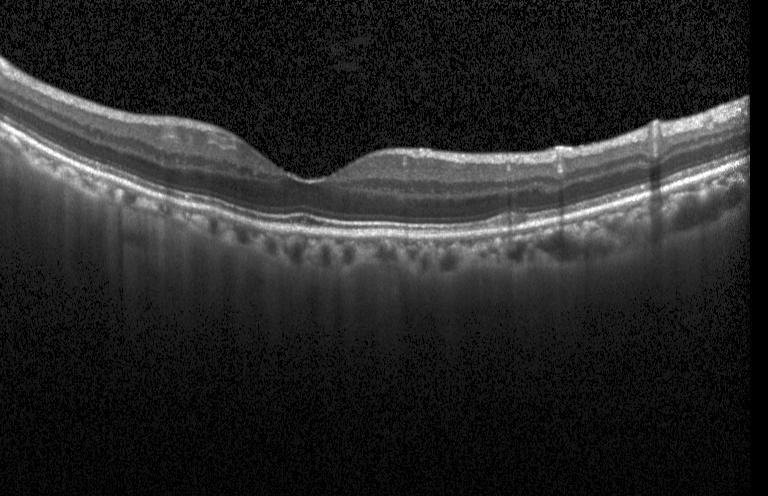

Spectral-domain OCT B-scan: neither choroidal neovascularization, diabetic macular edema, nor drusen.